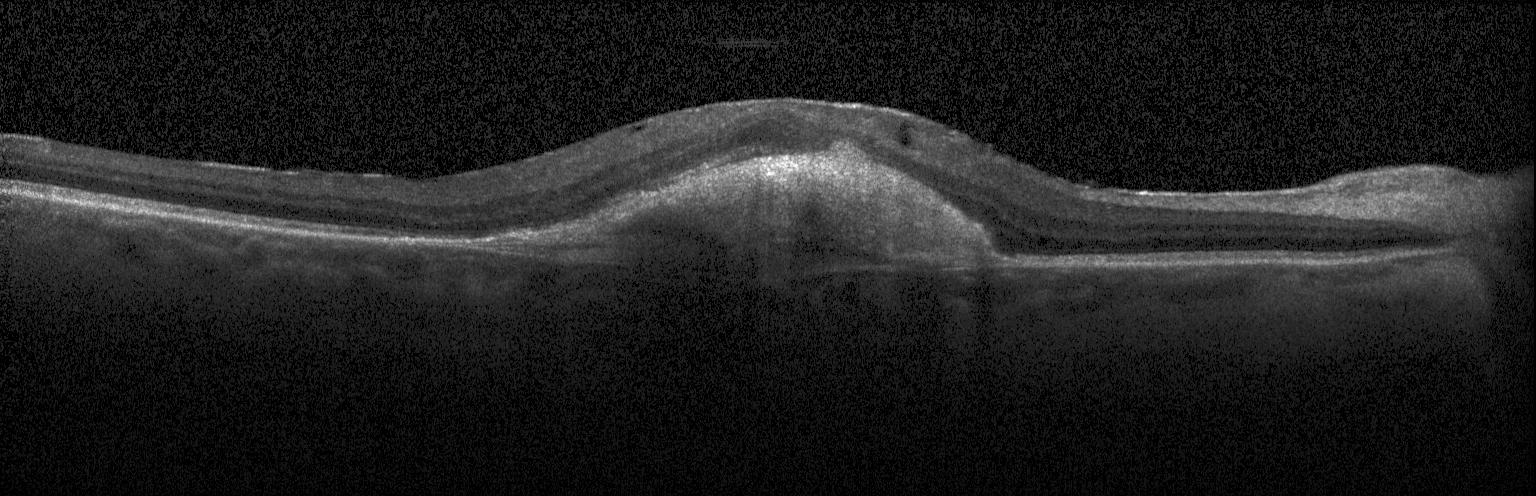

OCT B-scan · Heidelberg Spectralis — OCT finding: a choroidal neovascular membrane.